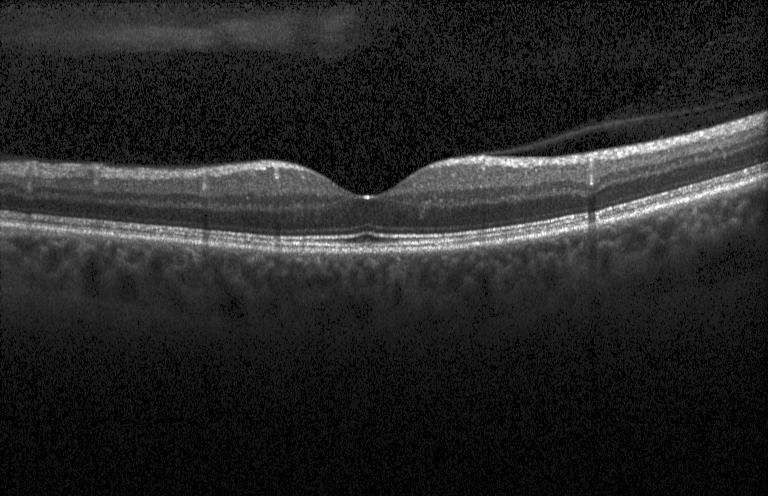
OCT finding: neither choroidal neovascularization, diabetic macular edema, nor drusen.